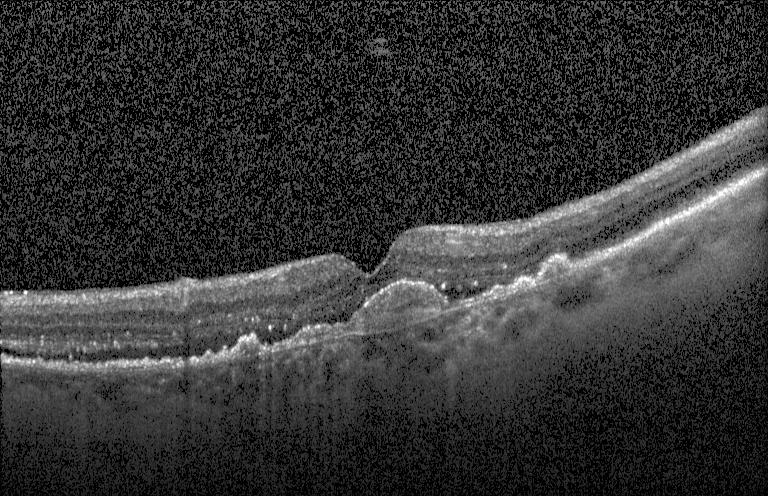 Retinal OCT B-scan.
This B-scan demonstrates a choroidal neovascular membrane.